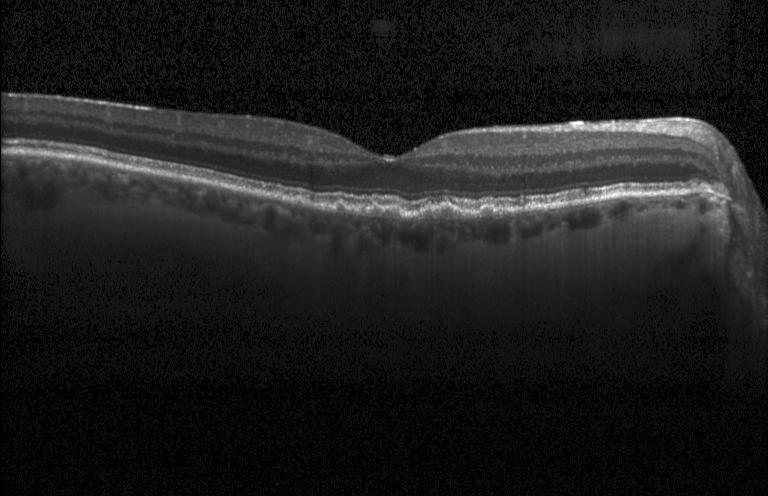

Optical coherence tomography B-scan.
Dx: sub-RPE drusenoid deposits.